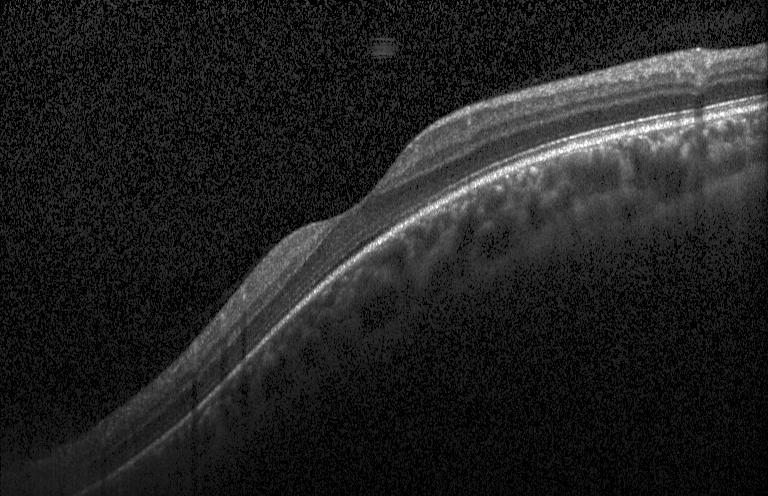
Horizontal scan through the fovea; Heidelberg Spectralis; retinal OCT B-scan
Macular OCT: neither choroidal neovascularization, diabetic macular edema, nor drusen.